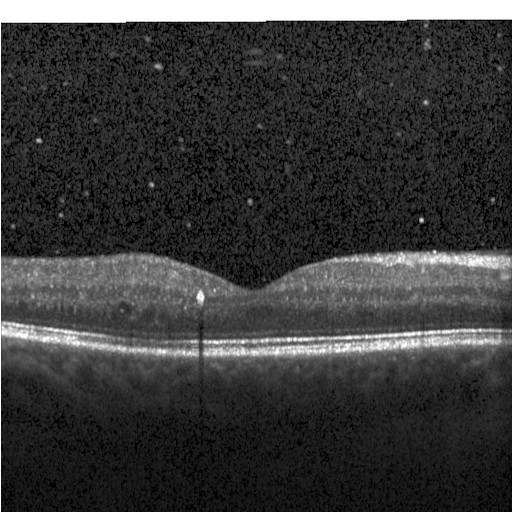

Heidelberg Spectralis · OCT line scan · SD-OCT
Diagnosis: diabetic macular edema (DME).